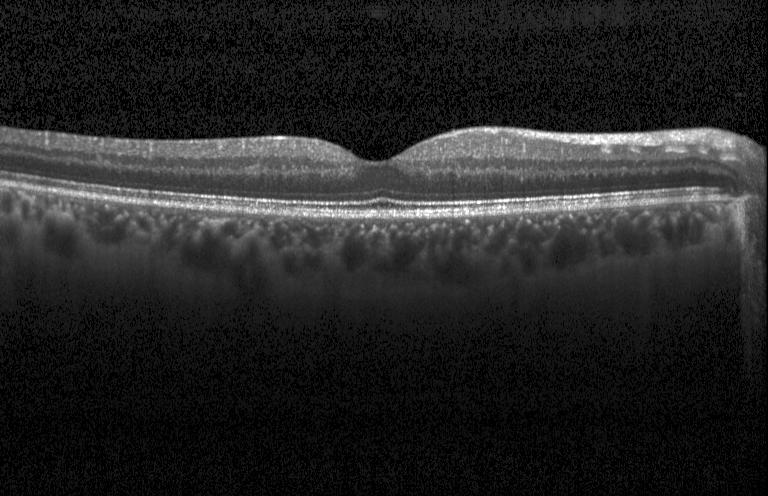 OCT line scan; SD-OCT; acquired on a Heidelberg Spectralis
Macular OCT: no choroidal neovascularization, no diabetic macular edema, and no drusen.